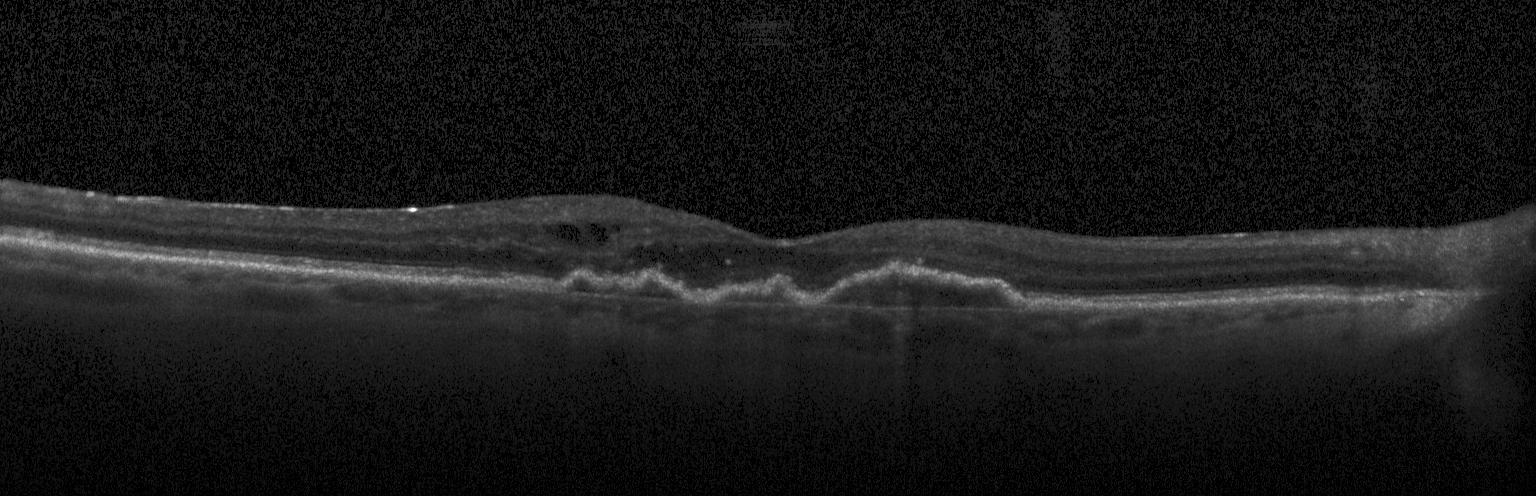

OCT finding: a choroidal neovascular membrane.